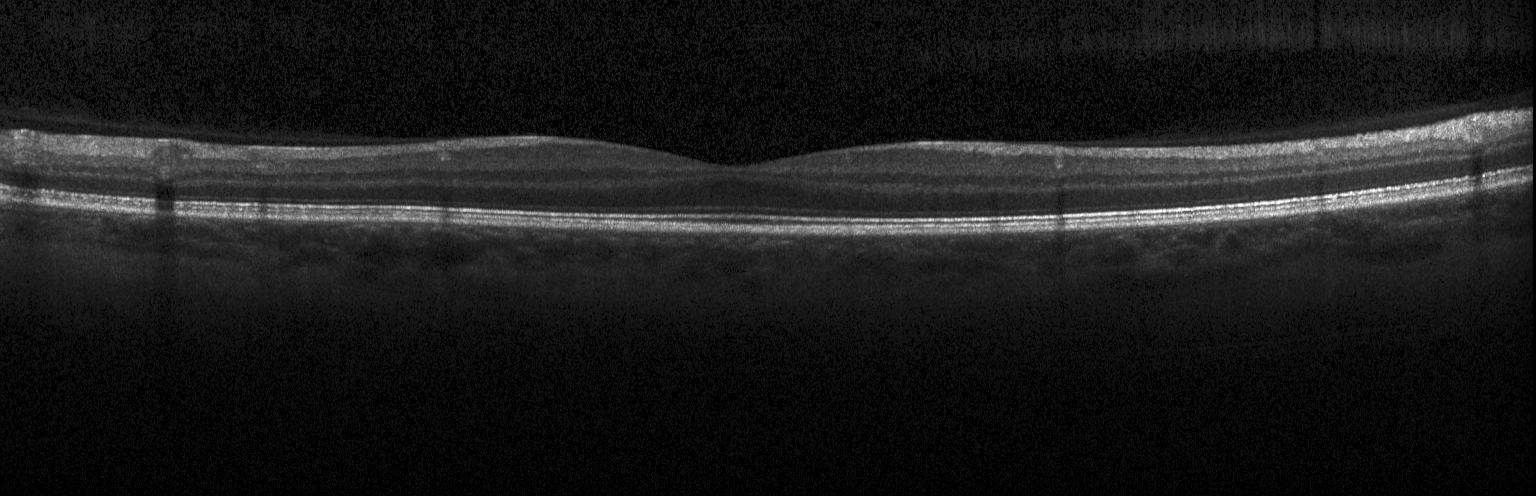

Spectral-domain OCT · instrument: Heidelberg Spectralis · retinal OCT cross-section
Finding: no choroidal neovascularization, no diabetic macular edema, and no drusen.